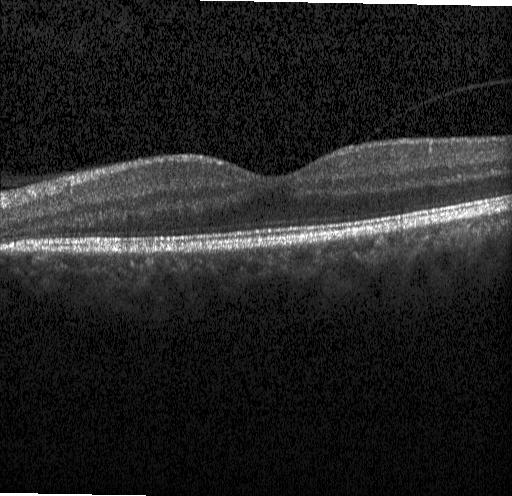 Macular OCT demonstrating no evidence of CNV, DME, or drusen.